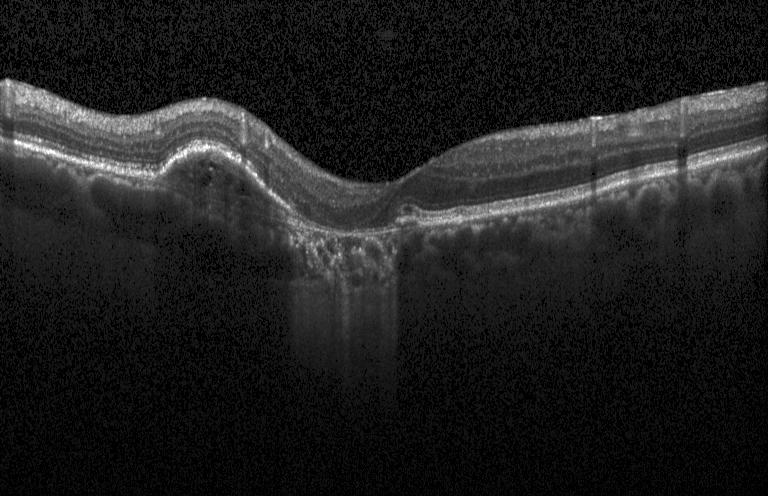 Diagnosis: a choroidal neovascular membrane.